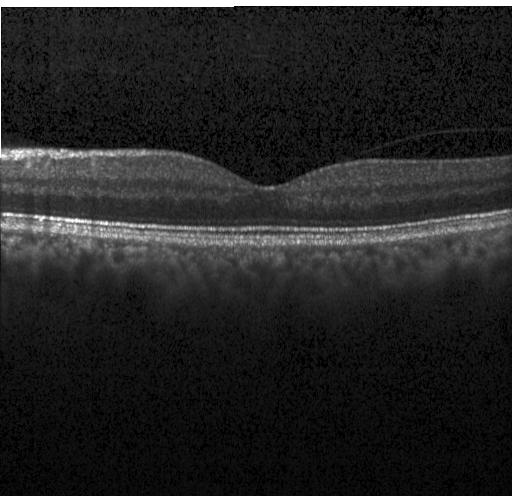 Horizontal scan through the fovea, SD-OCT, optical coherence tomography scan, Heidelberg Spectralis. Macular OCT: no evidence of CNV, DME, or drusen.